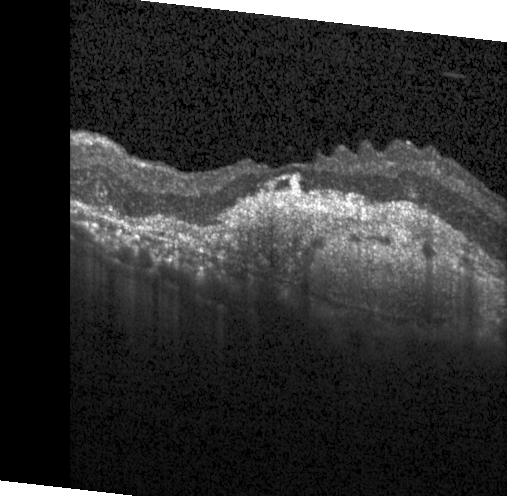

Macular OCT: CNV.